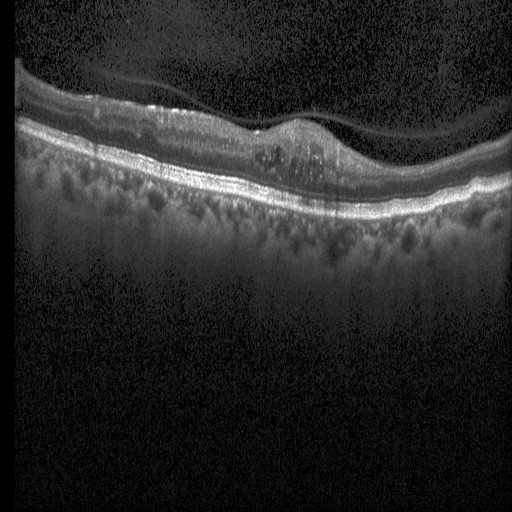

Finding: DME.